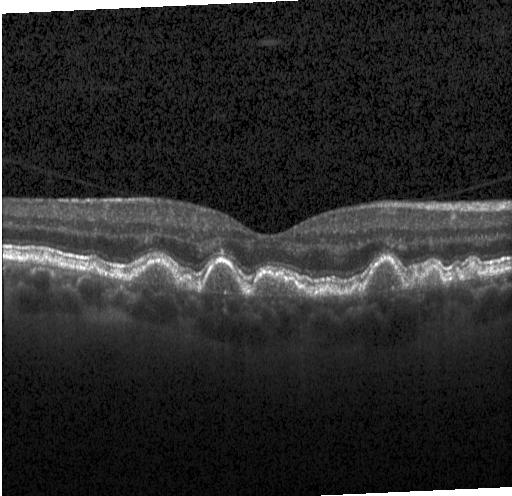 Retinal OCT cross-section, spectral-domain OCT
The scan shows drusen.